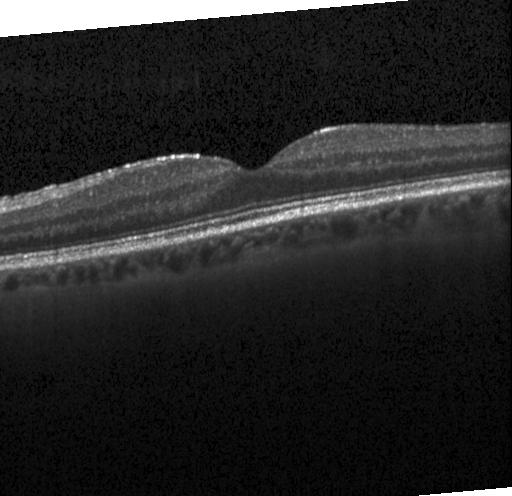
Through the macula, retinal OCT cross-section. Assessment: no choroidal neovascularization, diabetic macular edema, or drusen.